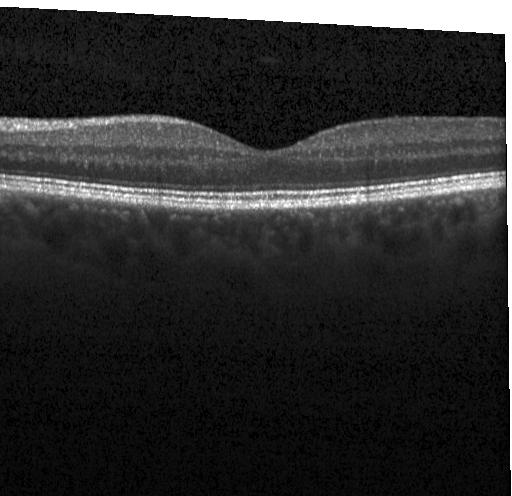

OCT B-scan; through the macula
Impression: no evidence of choroidal neovascularization, diabetic macular edema, or drusen.